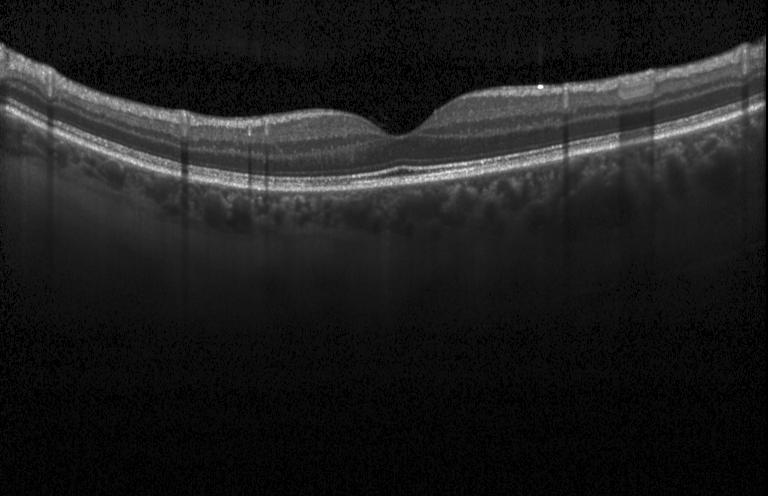 Optical coherence tomography scan, spectral-domain OCT, through the macula. Neither choroidal neovascularization, diabetic macular edema, nor drusen.